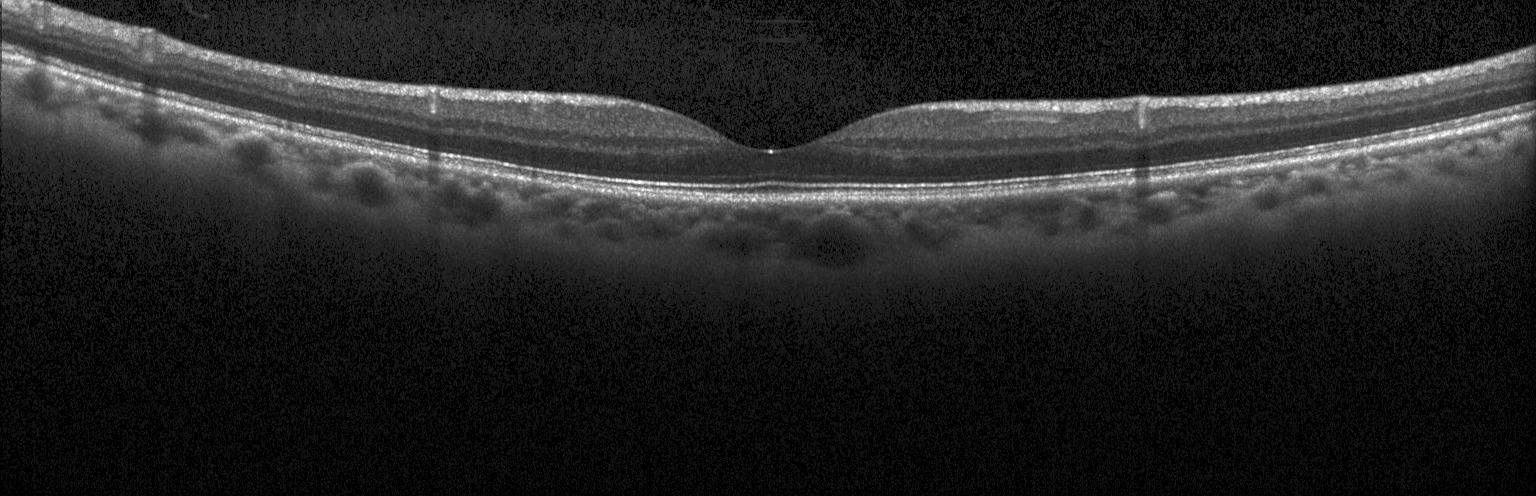 Fovea-centered, SD-OCT, OCT B-scan — Finding: no evidence of CNV, DME, or drusen.